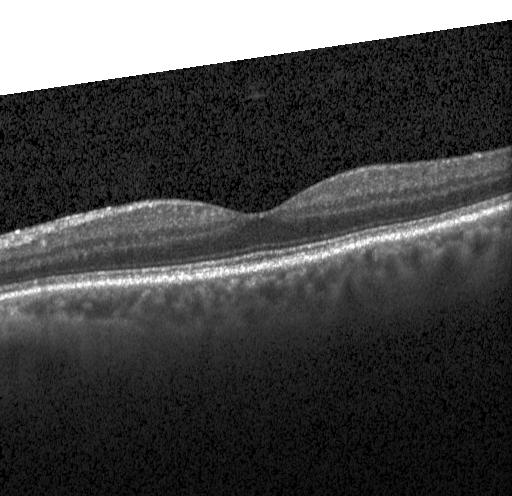

Dx: neither choroidal neovascularization, diabetic macular edema, nor drusen.